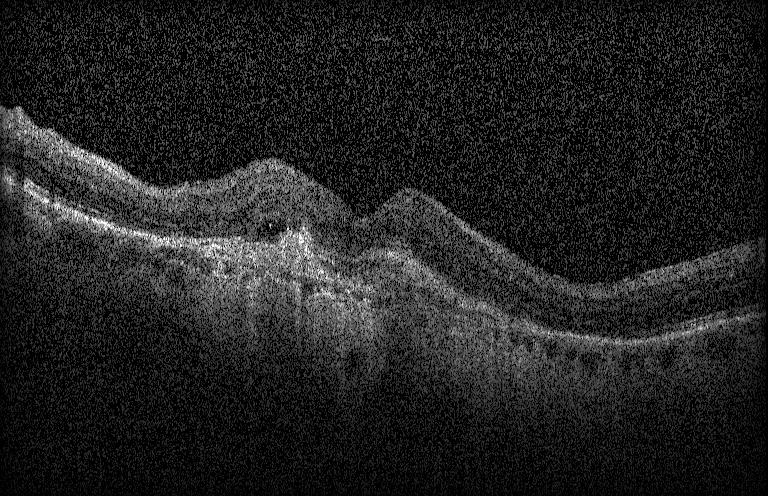
Fovea-centered; optical coherence tomography scan
Impression: a choroidal neovascular membrane.